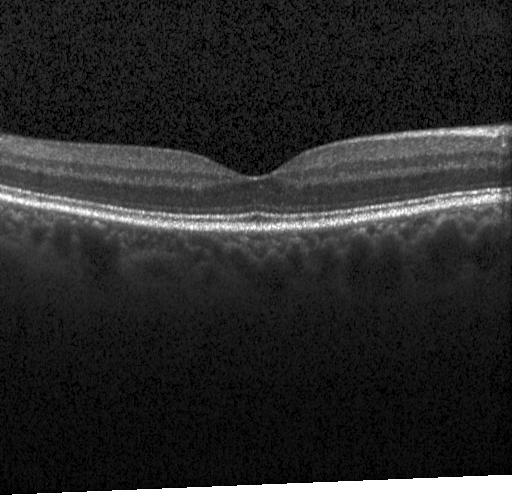

Impression: no evidence of choroidal neovascularization, diabetic macular edema, or drusen.